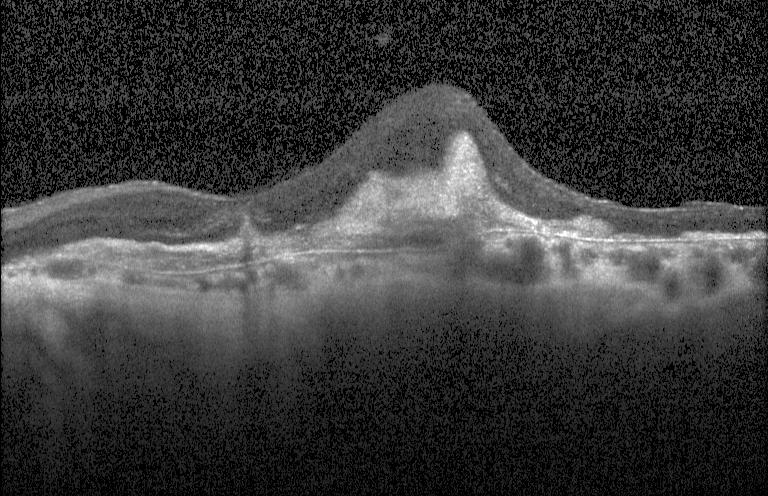
This B-scan demonstrates CNV.